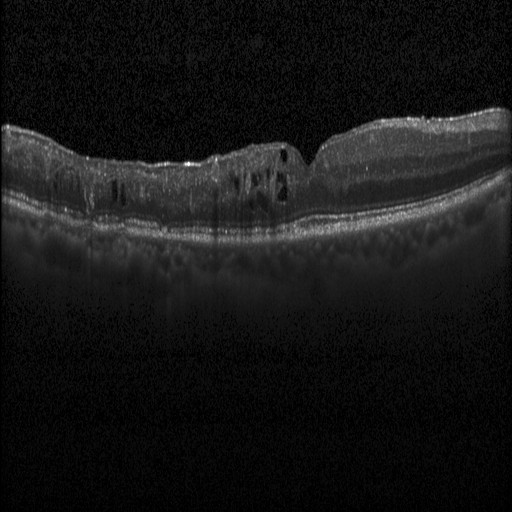
SD-OCT. OCT line scan. Through the macula.
Finding: diabetic macular edema (DME).